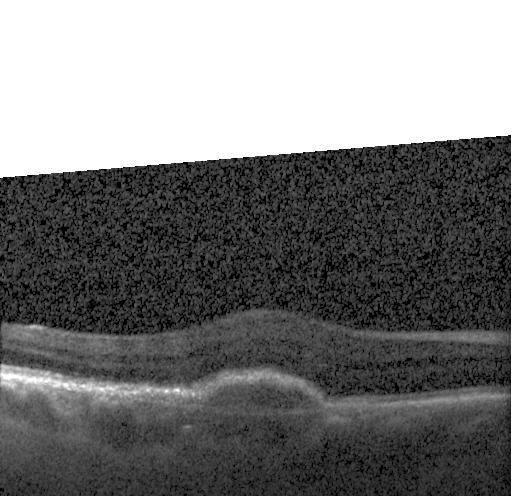

Diagnosis: a choroidal neovascular membrane.